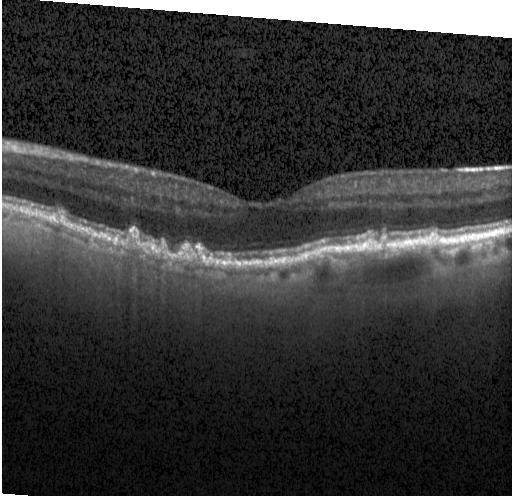

Diagnosis: multiple drusen.